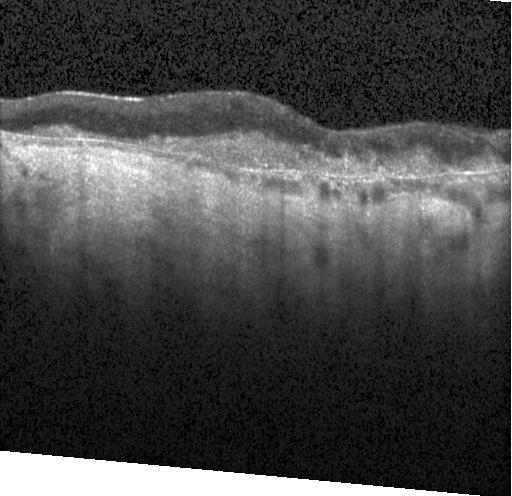
Impression: choroidal neovascularization.